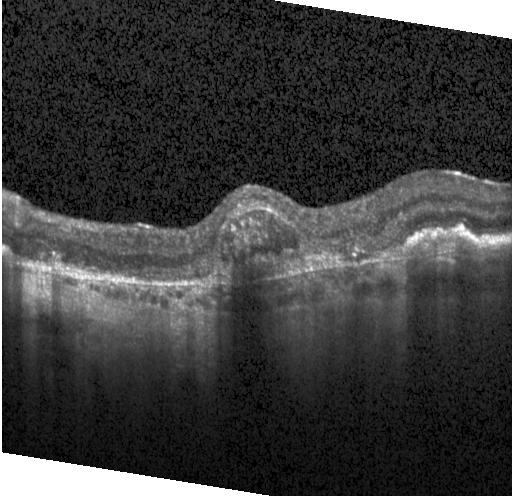

Through the macula · optical coherence tomography B-scan. This B-scan demonstrates a choroidal neovascular membrane.